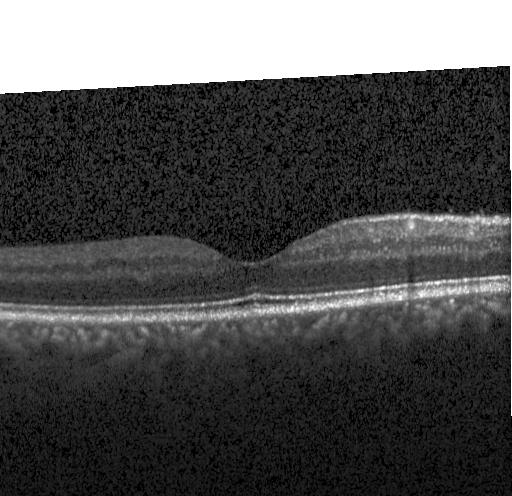 Macular OCT: no evidence of CNV, DME, or drusen.